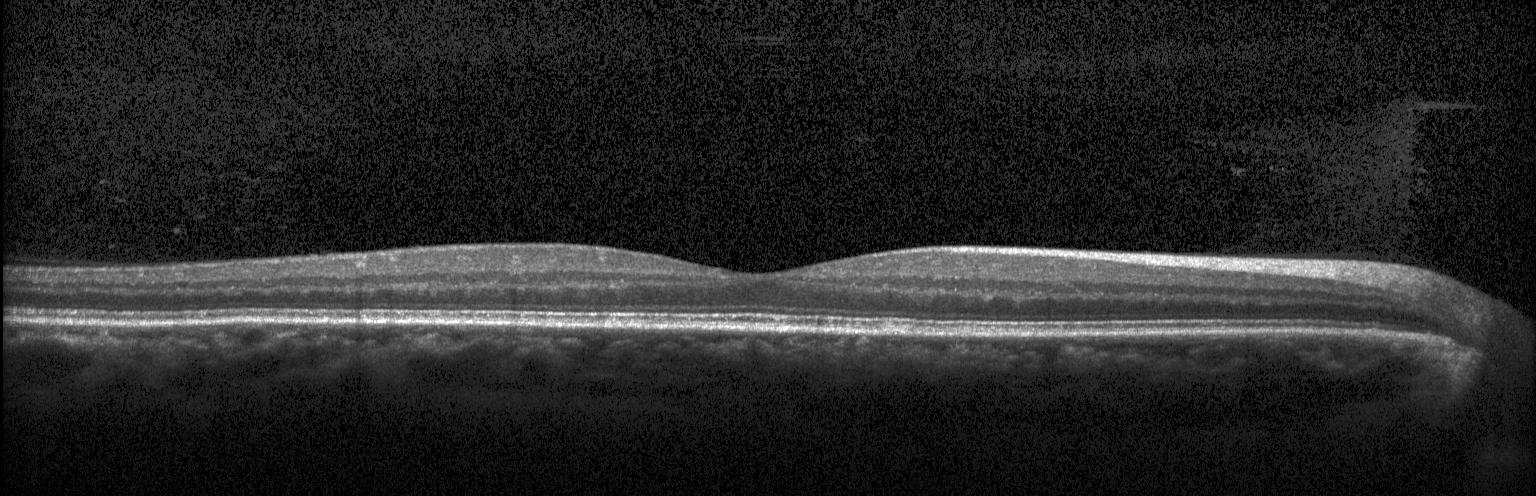
Retinal OCT cross-section; Heidelberg Spectralis OCT system. Finding: no choroidal neovascularization, no diabetic macular edema, and no drusen.